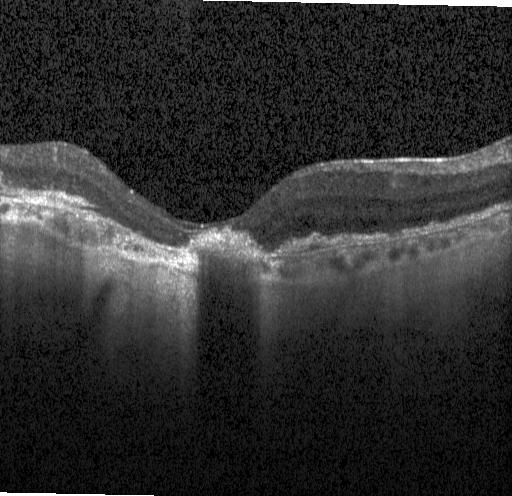
Spectral-domain OCT, OCT line scan, horizontal scan through the fovea.
Finding: choroidal neovascularization (CNV).